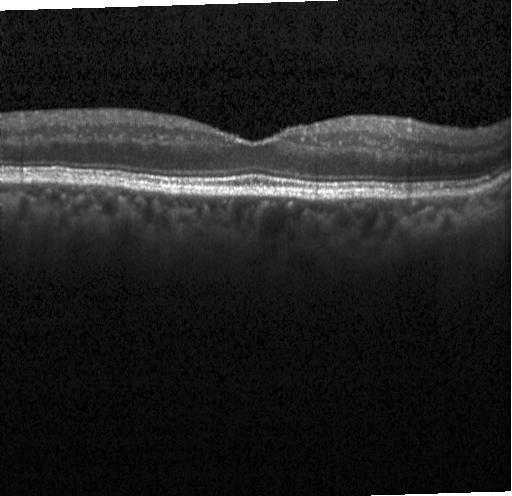

OCT finding: no choroidal neovascularization, no diabetic macular edema, and no drusen.